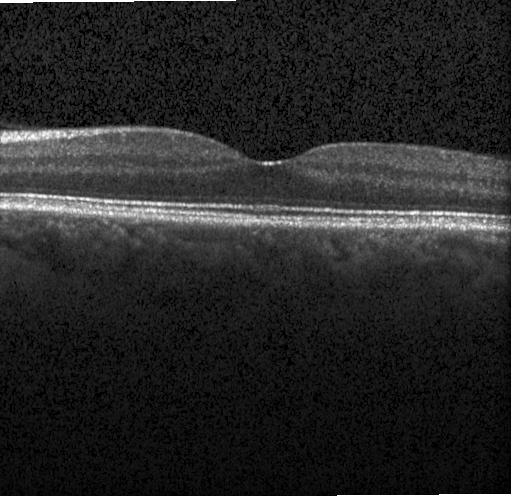

The scan shows no choroidal neovascularization, no diabetic macular edema, and no drusen.